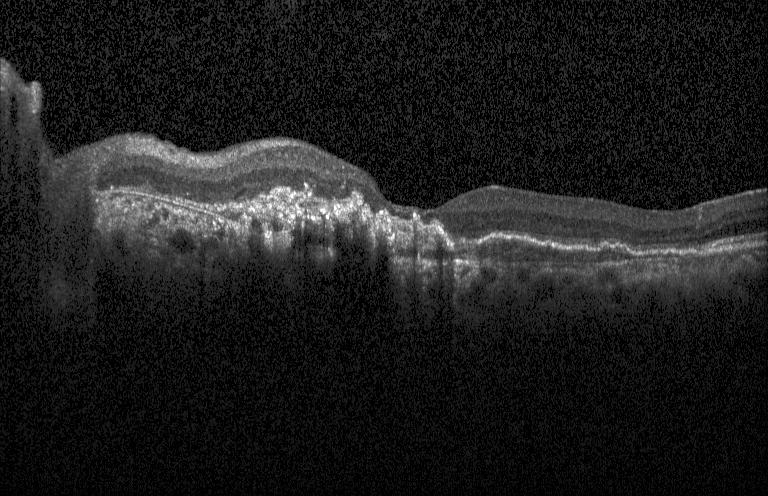
Retinal OCT B-scan.
This B-scan demonstrates CNV.